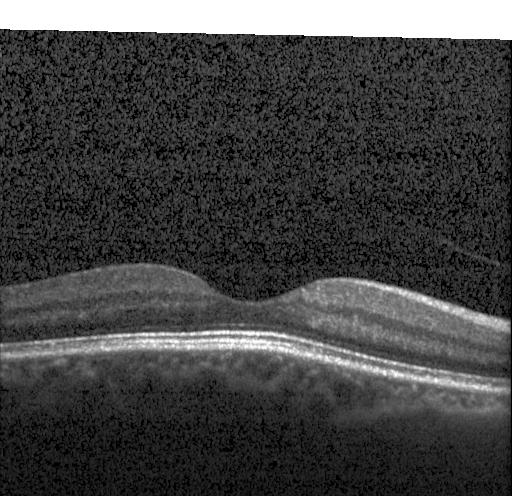
Through the macula. SD-OCT. Retinal OCT cross-section — Assessment: no evidence of choroidal neovascularization, diabetic macular edema, or drusen.